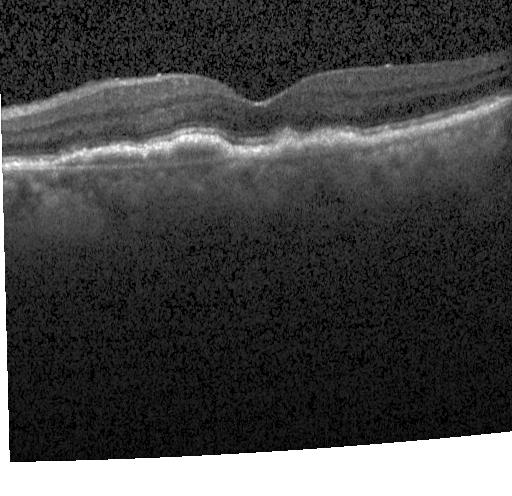
Retinal OCT B-scan · spectral-domain optical coherence tomography. Finding: choroidal neovascularization (CNV).